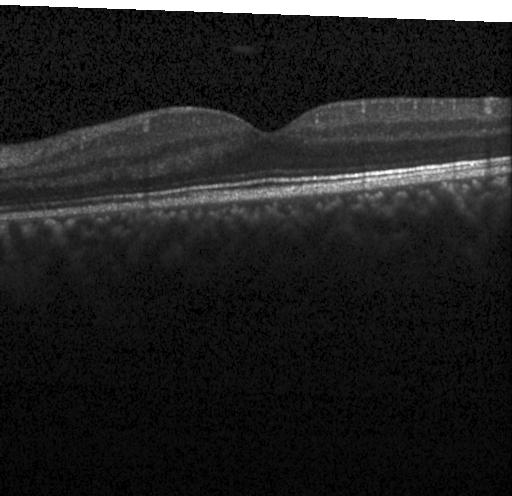

Spectral-domain optical coherence tomography; optical coherence tomography scan; Heidelberg Spectralis — Diagnosis: neither choroidal neovascularization, diabetic macular edema, nor drusen.